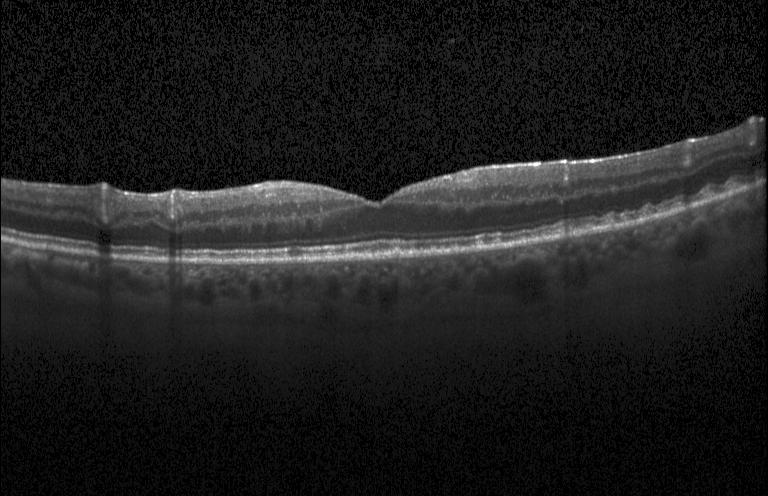

Diagnosis: neither choroidal neovascularization, diabetic macular edema, nor drusen.